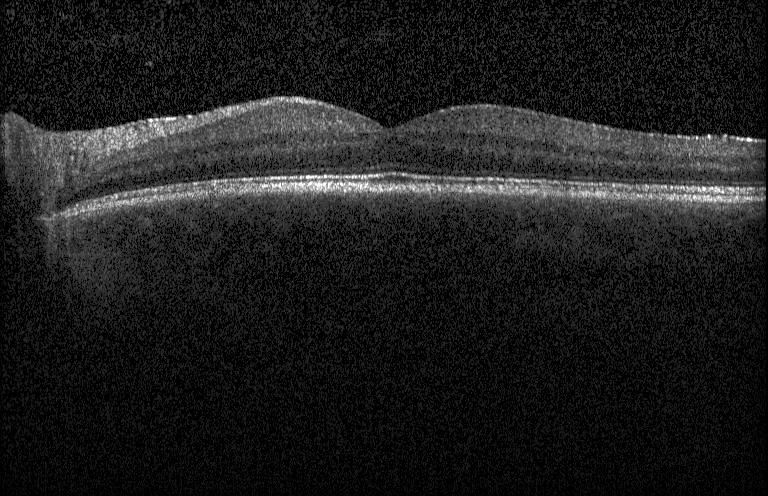
OCT B-scan. Finding: no choroidal neovascularization, diabetic macular edema, or drusen.